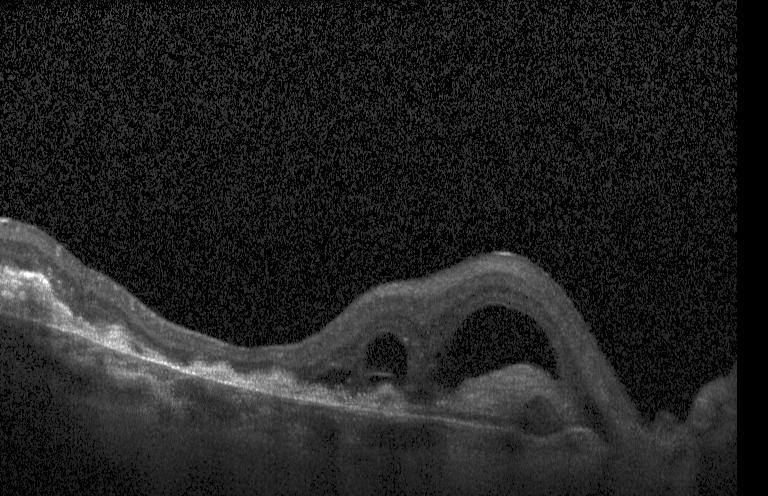 Optical coherence tomography B-scan · fovea-centered
The scan shows choroidal neovascularization (CNV).